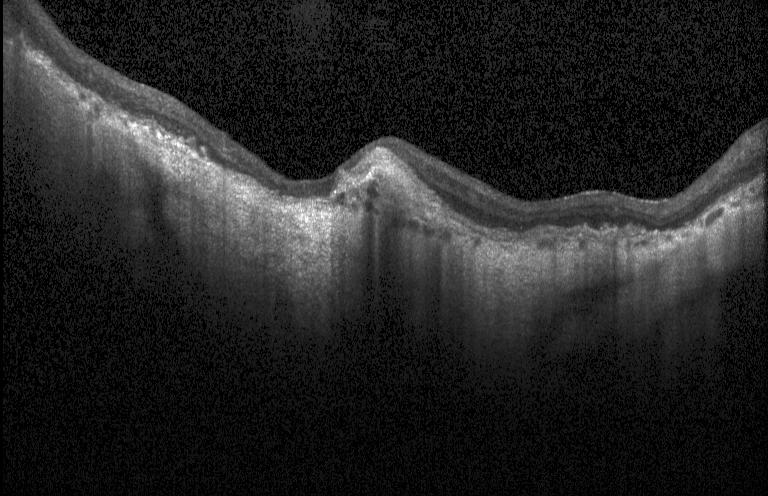

Fovea-centered; OCT line scan
The scan shows a choroidal neovascular membrane.